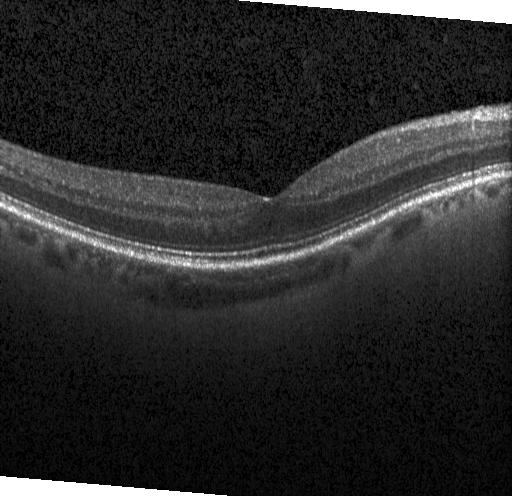

Spectral-domain optical coherence tomography. Heidelberg Spectralis OCT system. Horizontal scan through the fovea. Optical coherence tomography scan
The scan shows no choroidal neovascularization, diabetic macular edema, or drusen.